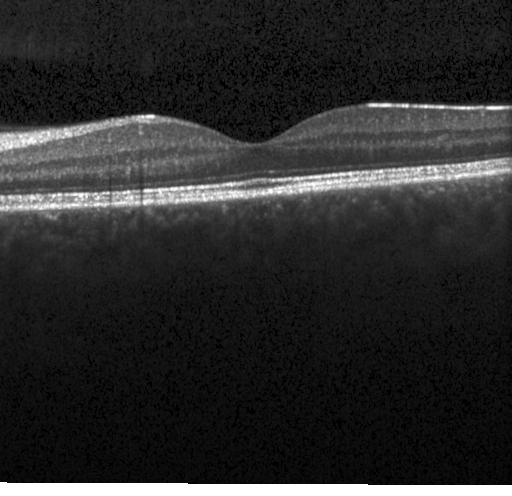
OCT line scan. Centered on the fovea. Heidelberg Spectralis OCT system. Finding: no choroidal neovascularization, no diabetic macular edema, and no drusen.